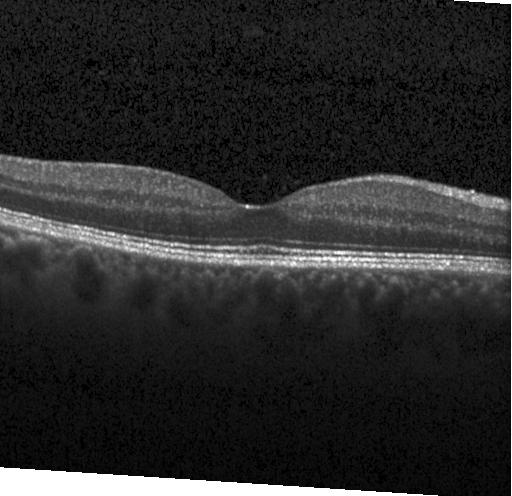 OCT finding: no evidence of choroidal neovascularization, diabetic macular edema, or drusen.